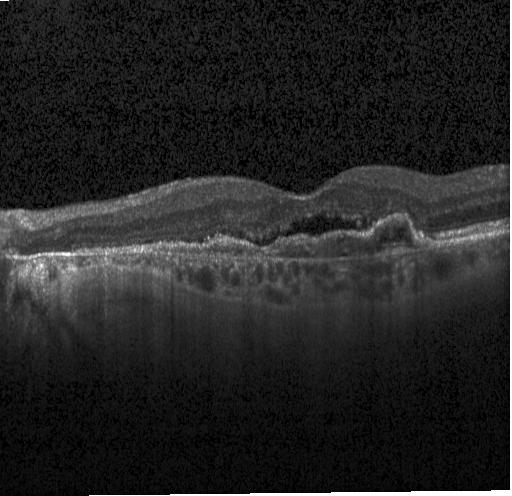

OCT finding: choroidal neovascularization (CNV).